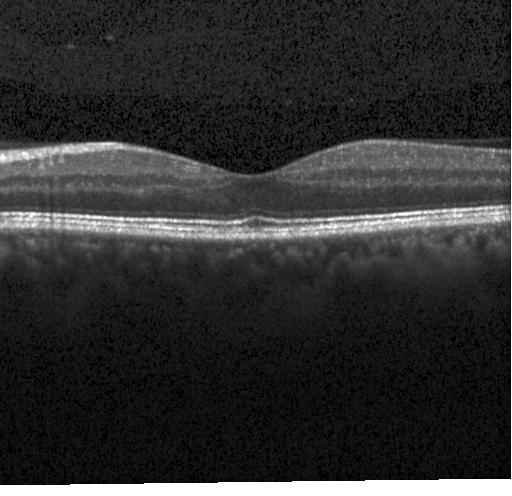 Heidelberg Spectralis OCT system, OCT B-scan, SD-OCT. Neither choroidal neovascularization, diabetic macular edema, nor drusen.